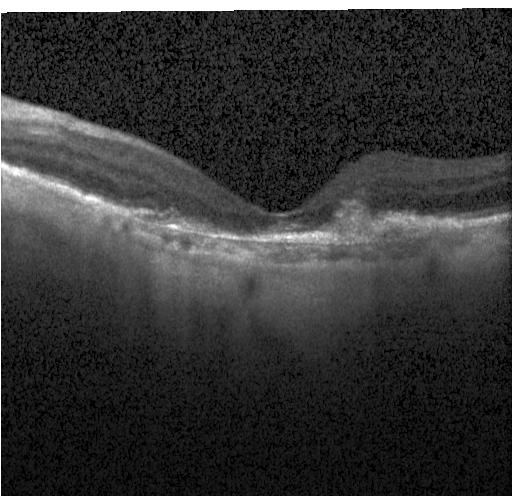

This B-scan demonstrates a choroidal neovascular membrane.